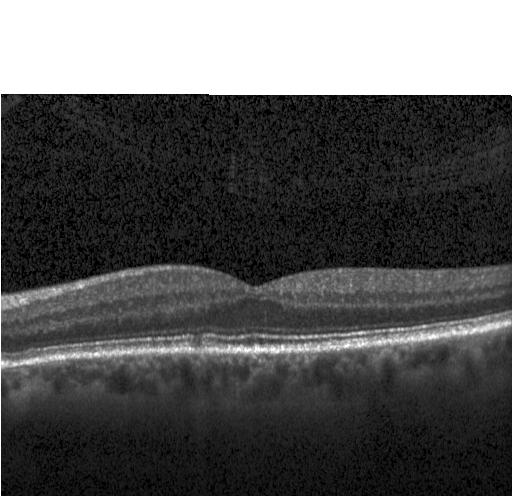 Impression: no choroidal neovascularization, no diabetic macular edema, and no drusen.